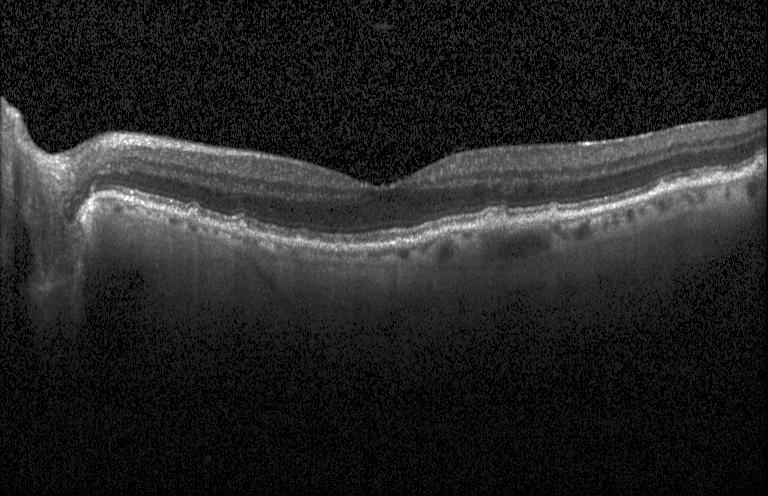 Macular OCT demonstrating multiple drusen.